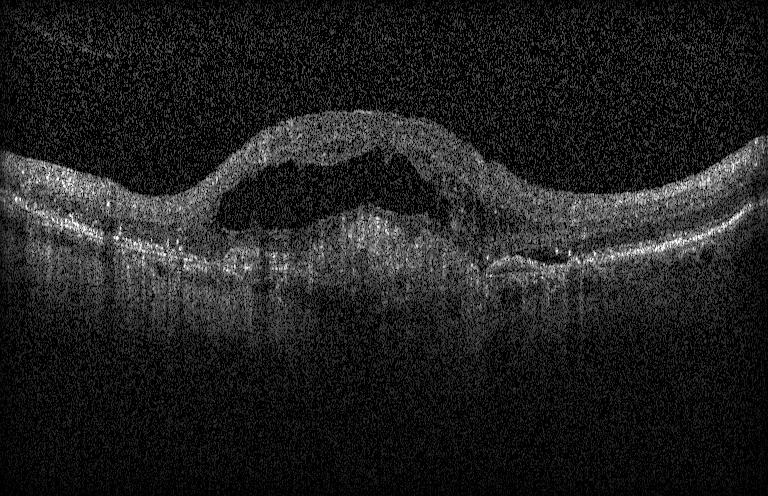

Heidelberg Spectralis; horizontal scan through the fovea; OCT line scan. The scan shows choroidal neovascularization.